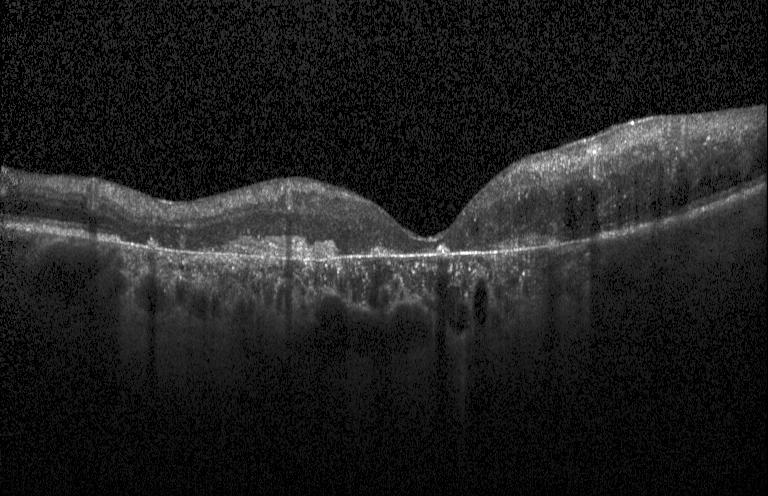 The scan shows choroidal neovascularization (CNV).